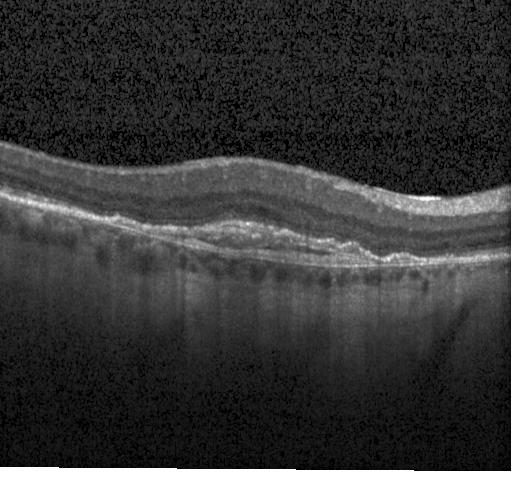 OCT scan showing a choroidal neovascular membrane.